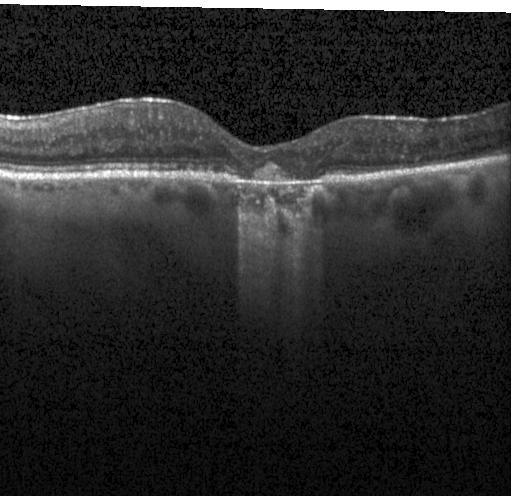 OCT B-scan. Diagnosis: a choroidal neovascular membrane.